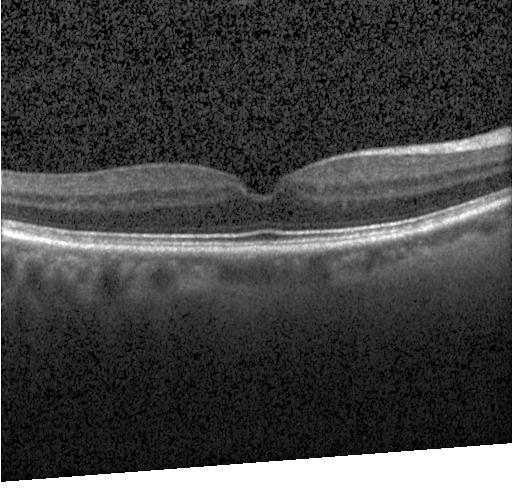

OCT line scan.
Diagnosis: no choroidal neovascularization, diabetic macular edema, or drusen.